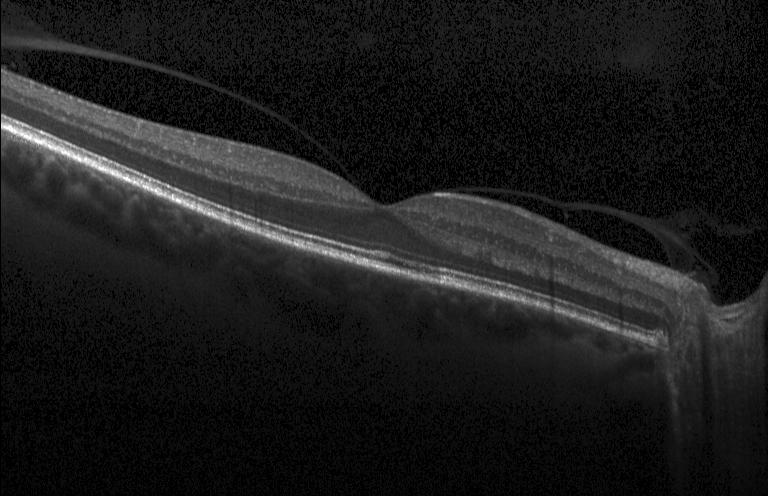 Macular scan, SD-OCT, Heidelberg Spectralis, OCT line scan.
Finding: no choroidal neovascularization, diabetic macular edema, or drusen.